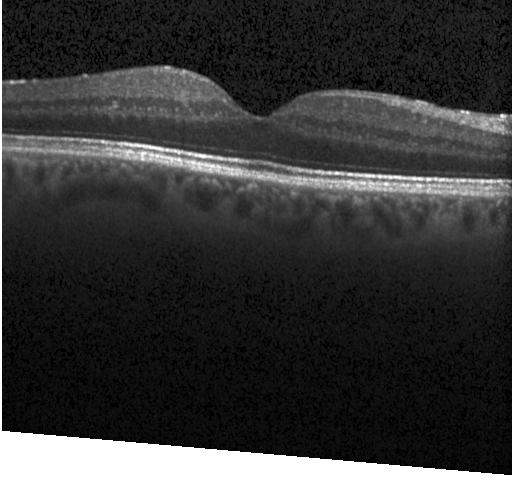
Optical coherence tomography B-scan.
The scan shows no evidence of choroidal neovascularization, diabetic macular edema, or drusen.